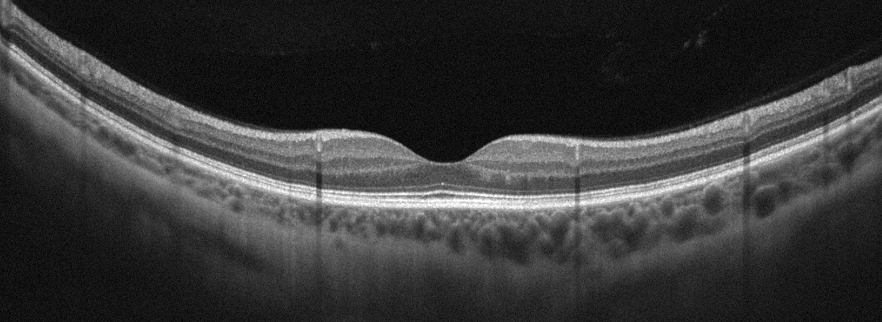

Oculus sinister. OCT B-scan
Impression: no AMD, DME, ERM, RAO, RVO, or VID.